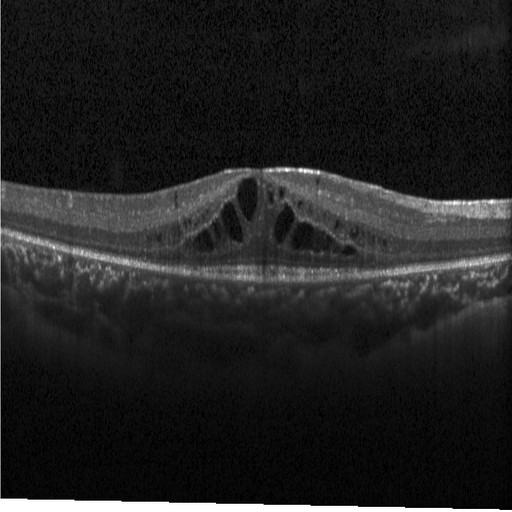 SD-OCT · instrument: Heidelberg Spectralis · fovea-centered · retinal OCT cross-section — Finding: diabetic macular edema (DME).